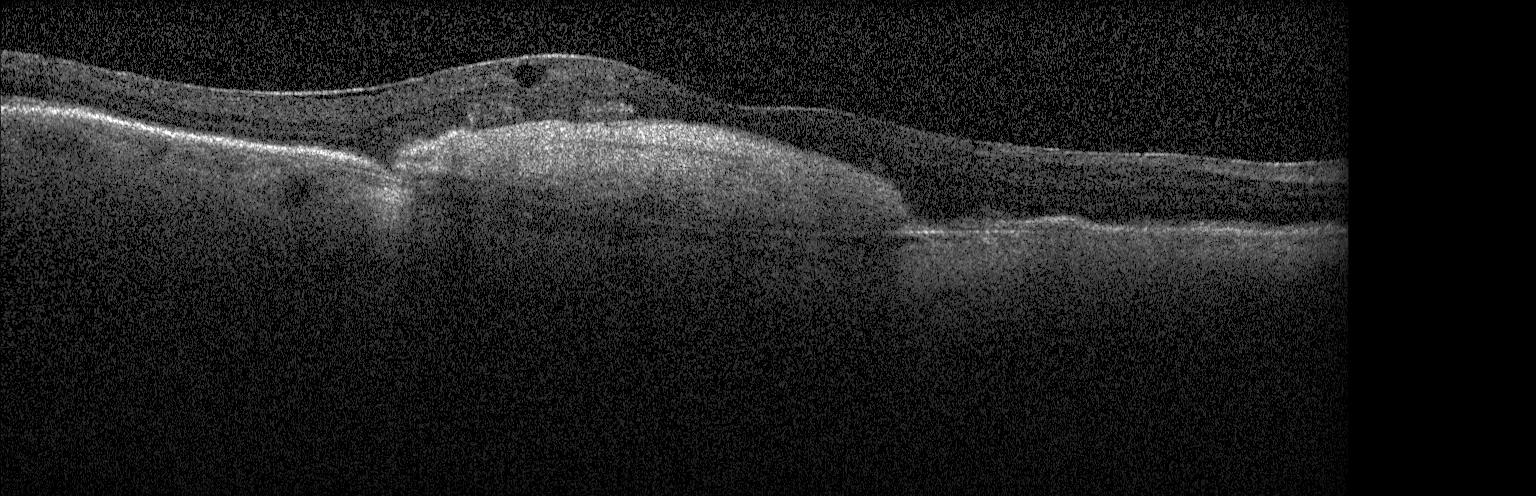
OCT scan showing a choroidal neovascular membrane.